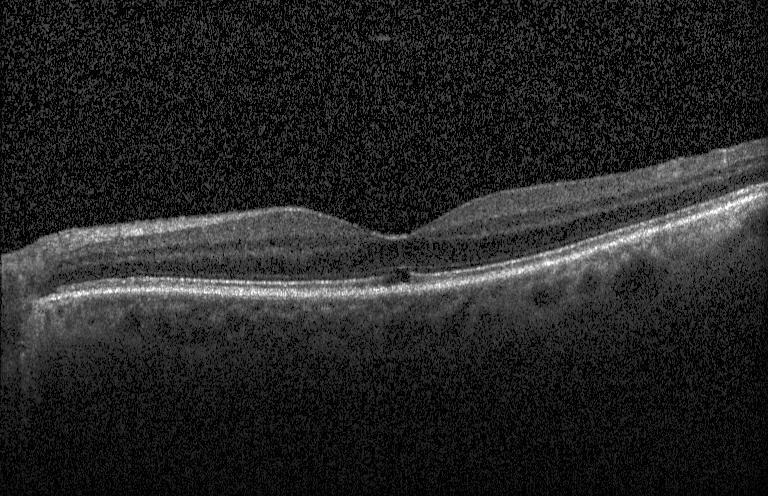

Through the macula · retinal OCT B-scan.
This B-scan demonstrates neither CNV, DME, nor drusen.